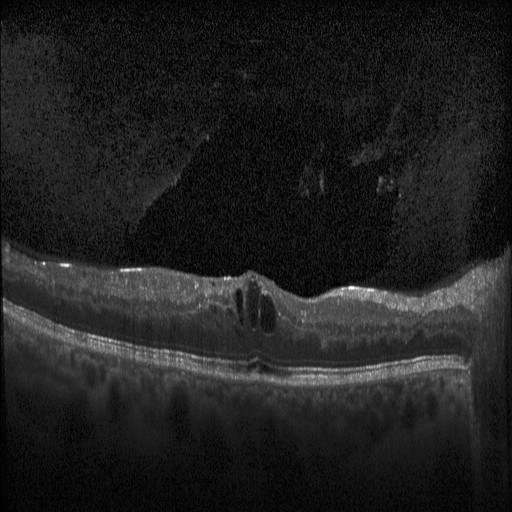
Optical coherence tomography scan.
Finding: diabetic macular edema (DME).